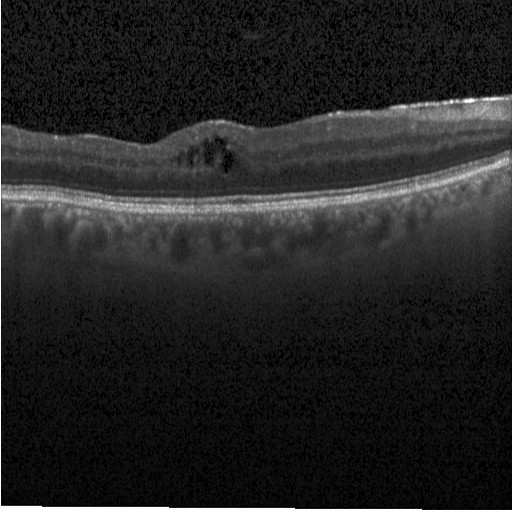
Finding: diabetic macular edema (DME).